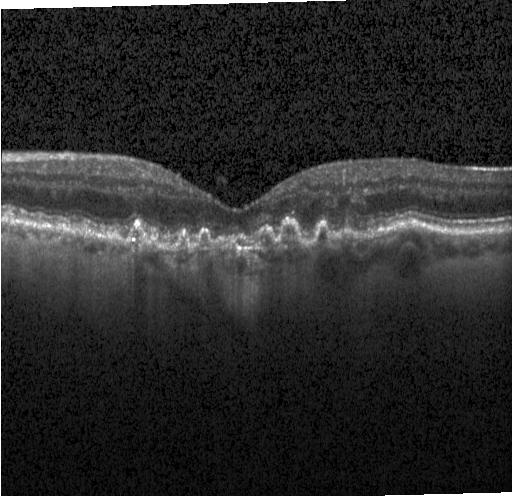

Centered on the fovea; Heidelberg Spectralis; retinal OCT B-scan
Dx: multiple drusen.